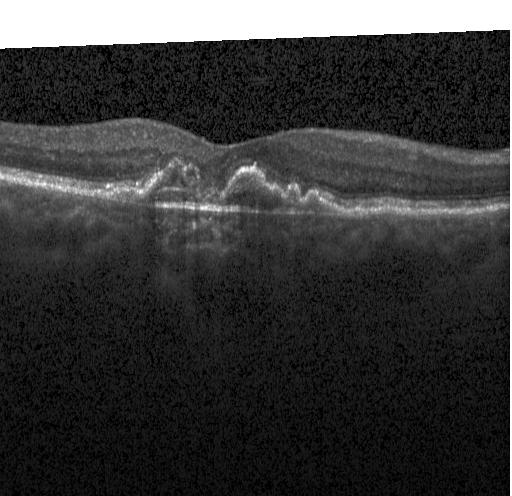

Acquired on a Heidelberg Spectralis, OCT line scan.
This B-scan demonstrates choroidal neovascularization (CNV).